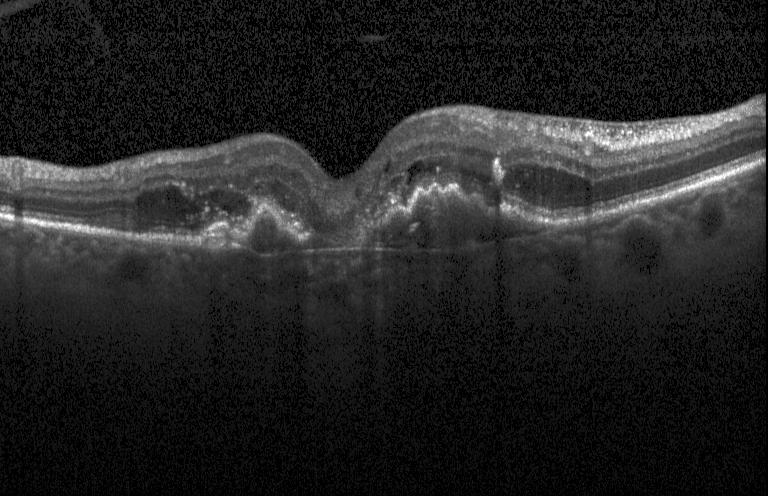

Impression: a choroidal neovascular membrane.